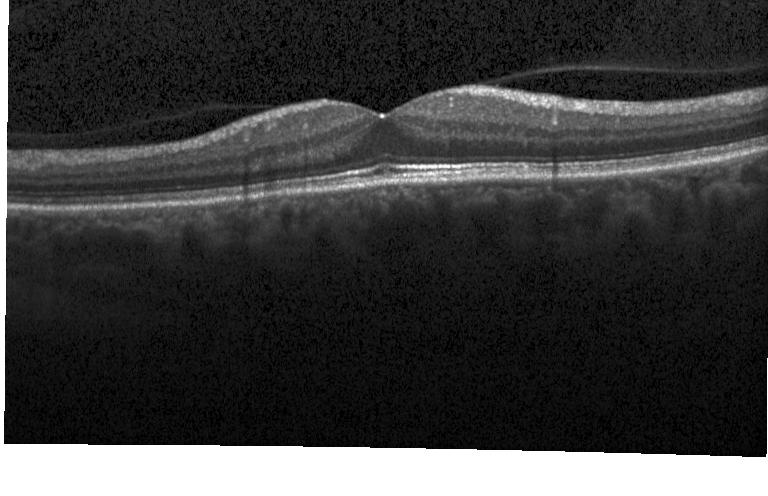
Impression: neither CNV, DME, nor drusen.